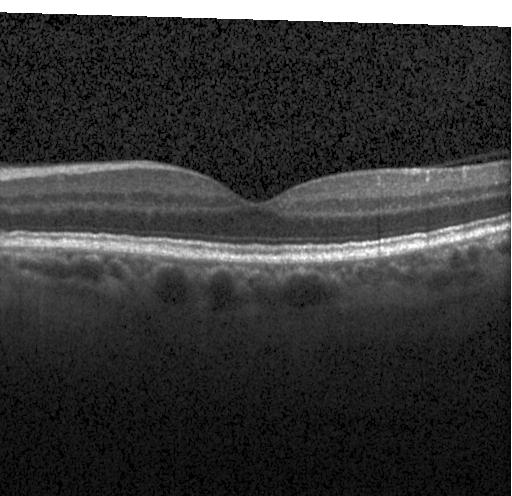 No CNV, no DME, and no drusen.